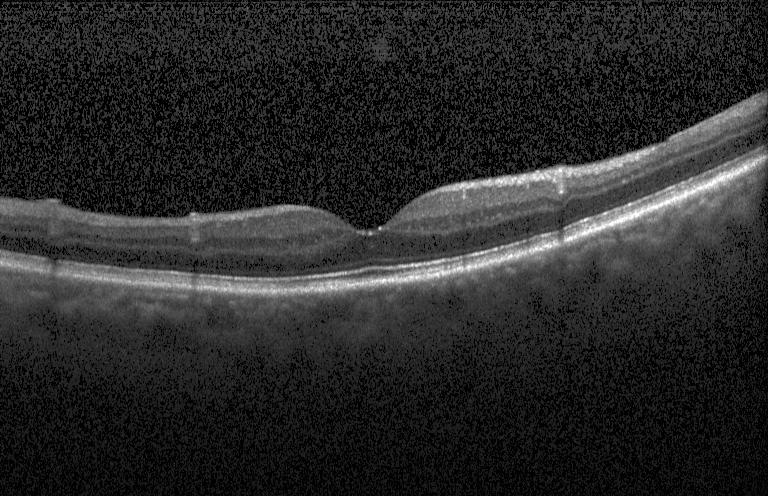
Optical coherence tomography B-scan — Impression: no choroidal neovascularization, diabetic macular edema, or drusen.